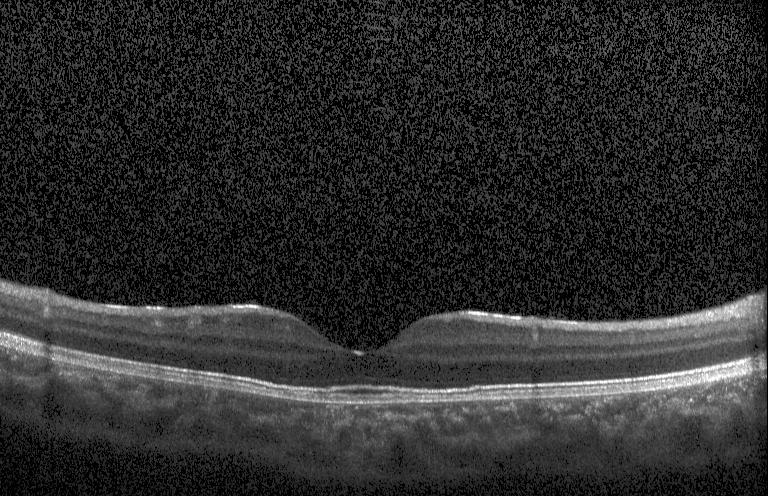 The scan shows no evidence of choroidal neovascularization, diabetic macular edema, or drusen.